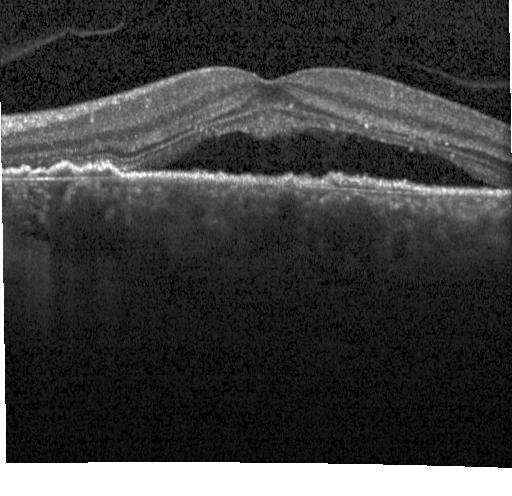 Impression: CNV.